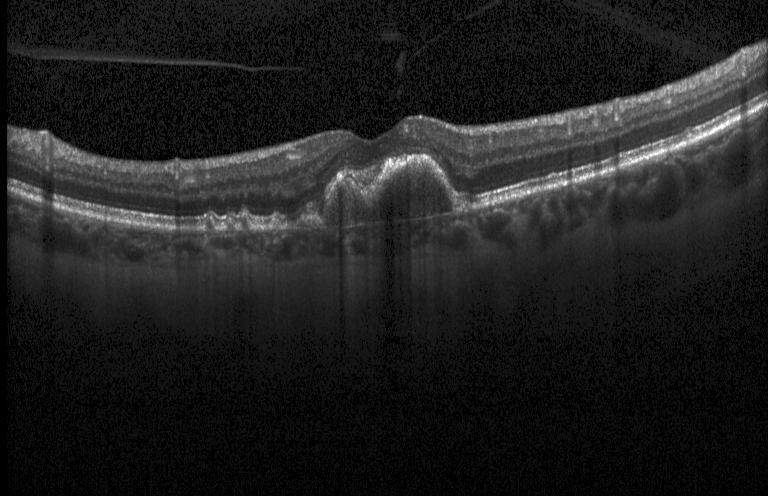

Macular OCT: choroidal neovascularization.